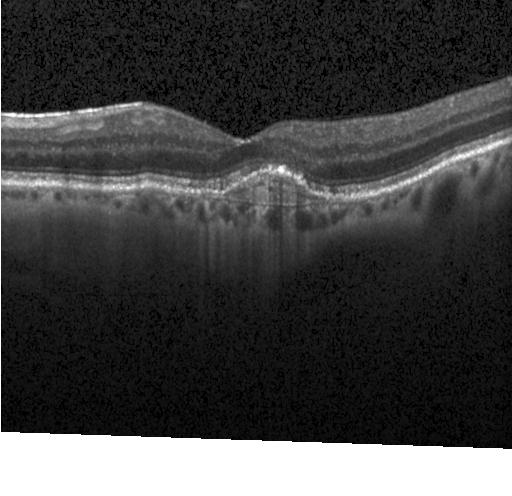 OCT B-scan; spectral-domain OCT — Macular OCT: CNV.